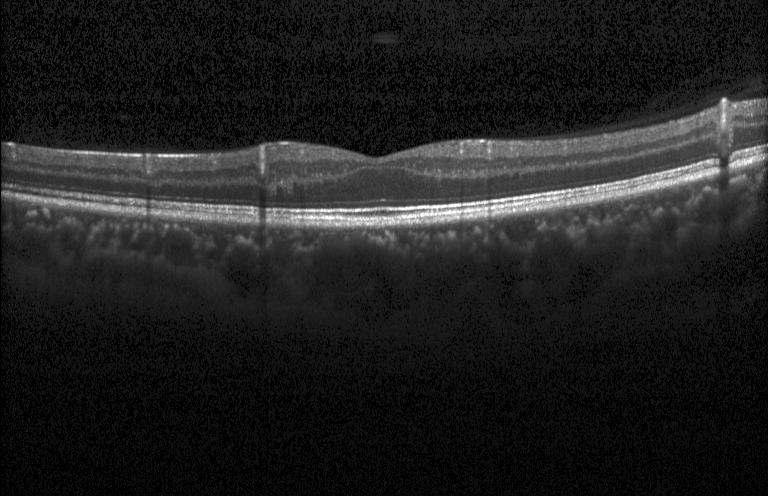 No CNV, DME, or drusen.